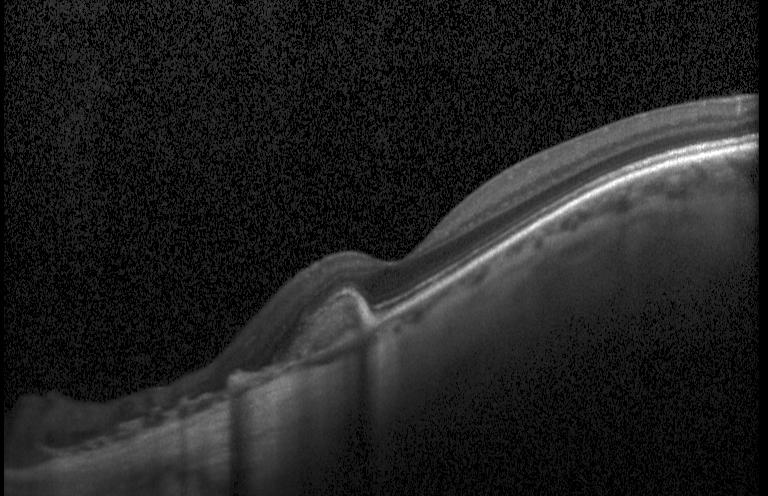

SD-OCT, optical coherence tomography scan, Heidelberg Spectralis.
A choroidal neovascular membrane.